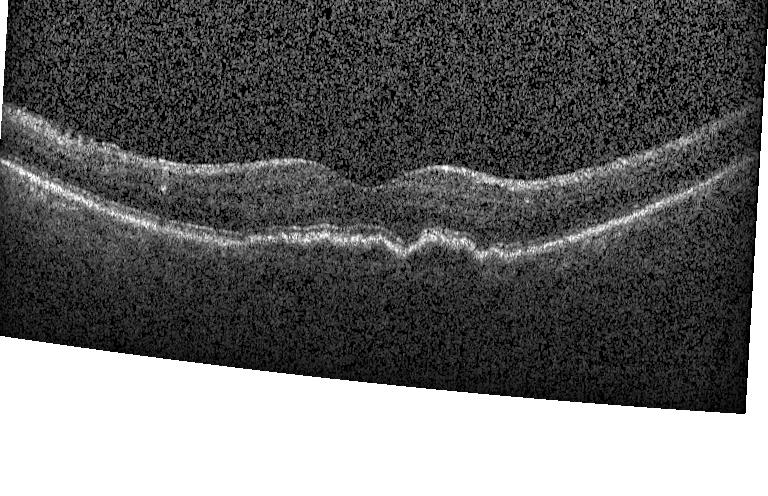 Spectral-domain OCT · horizontal scan through the fovea · retinal OCT cross-section
This B-scan demonstrates choroidal neovascularization.